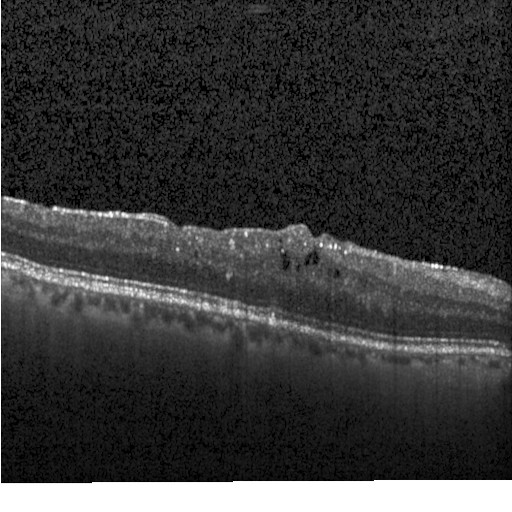

OCT B-scan. Heidelberg Spectralis OCT system
Dx: diabetic macular edema.